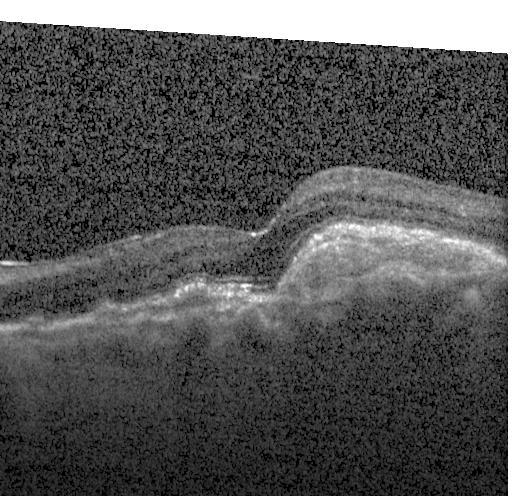 Optical coherence tomography scan. Spectral-domain optical coherence tomography. Instrument: Heidelberg Spectralis.
The scan shows choroidal neovascularization (CNV).